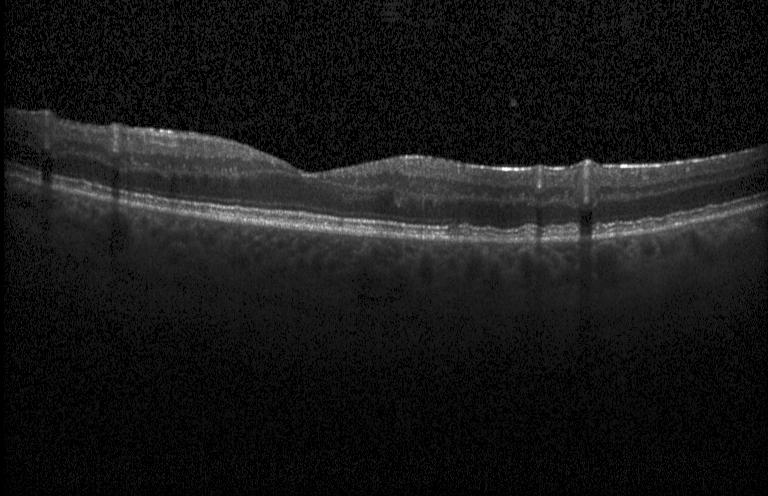

Finding: sub-RPE drusenoid deposits.